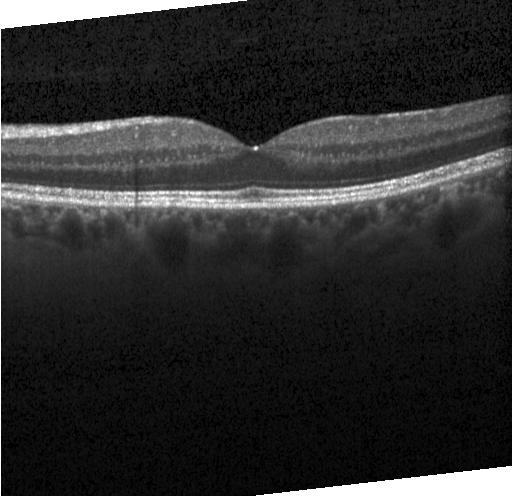 Retinal OCT cross-section; Heidelberg Spectralis OCT system; horizontal scan through the fovea — Diagnosis: no CNV, DME, or drusen.